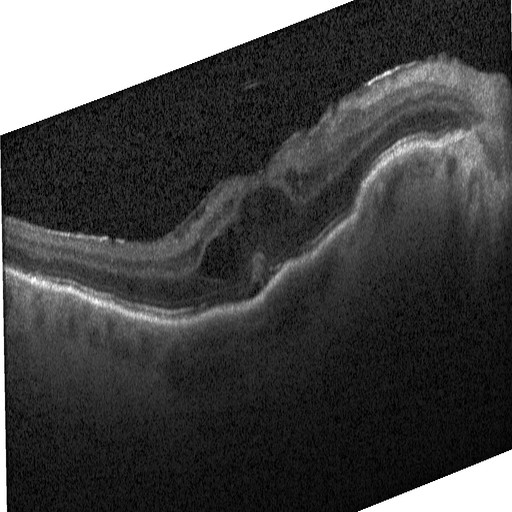
Spectral-domain optical coherence tomography; OCT B-scan; through the macula
Diagnosis: diabetic macular edema (DME).